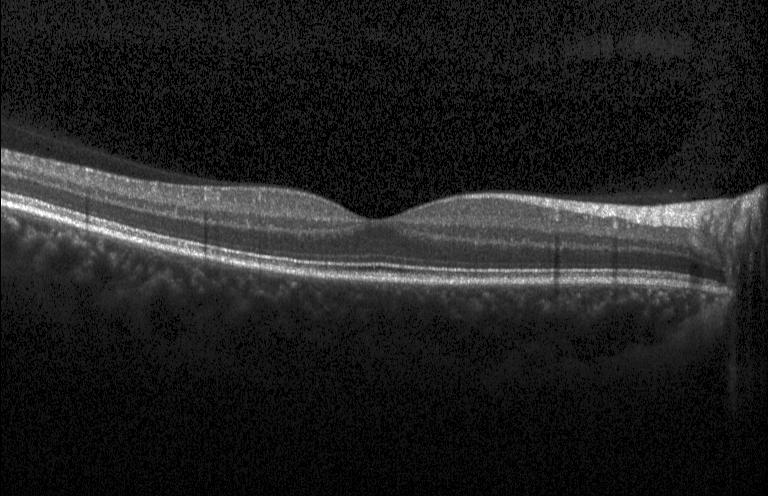 OCT finding: no CNV, DME, or drusen.